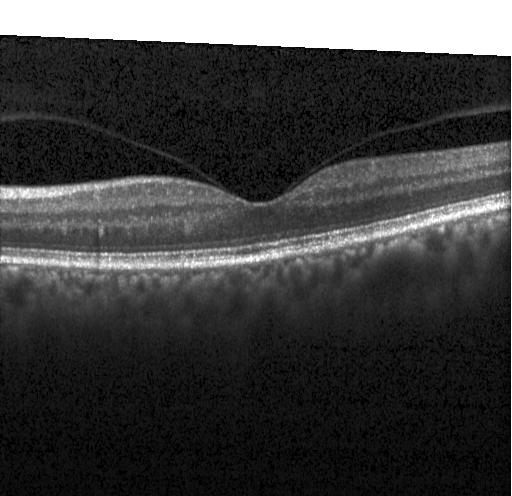

Optical coherence tomography scan.
Finding: no choroidal neovascularization, diabetic macular edema, or drusen.